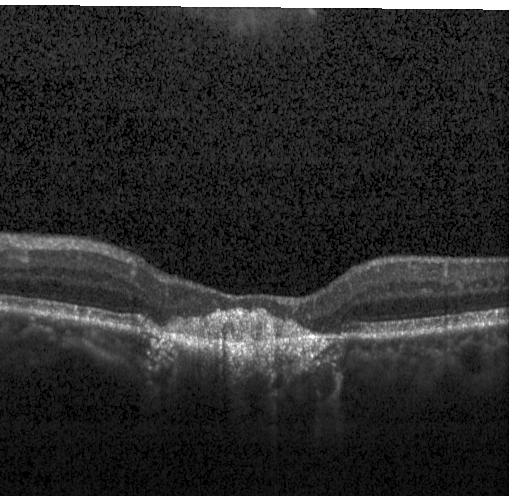 Centered on the fovea; OCT line scan
OCT finding: choroidal neovascularization.